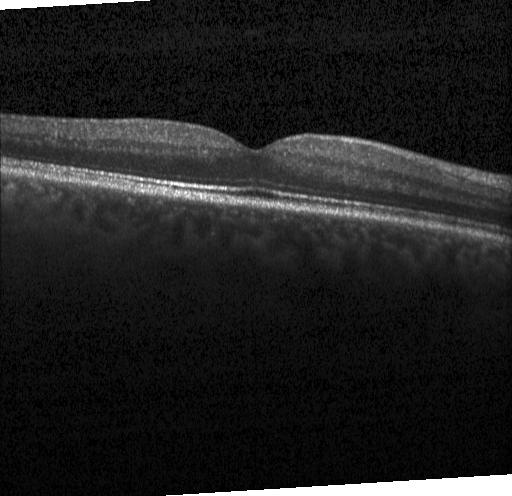

Optical coherence tomography scan — This B-scan demonstrates neither choroidal neovascularization, diabetic macular edema, nor drusen.